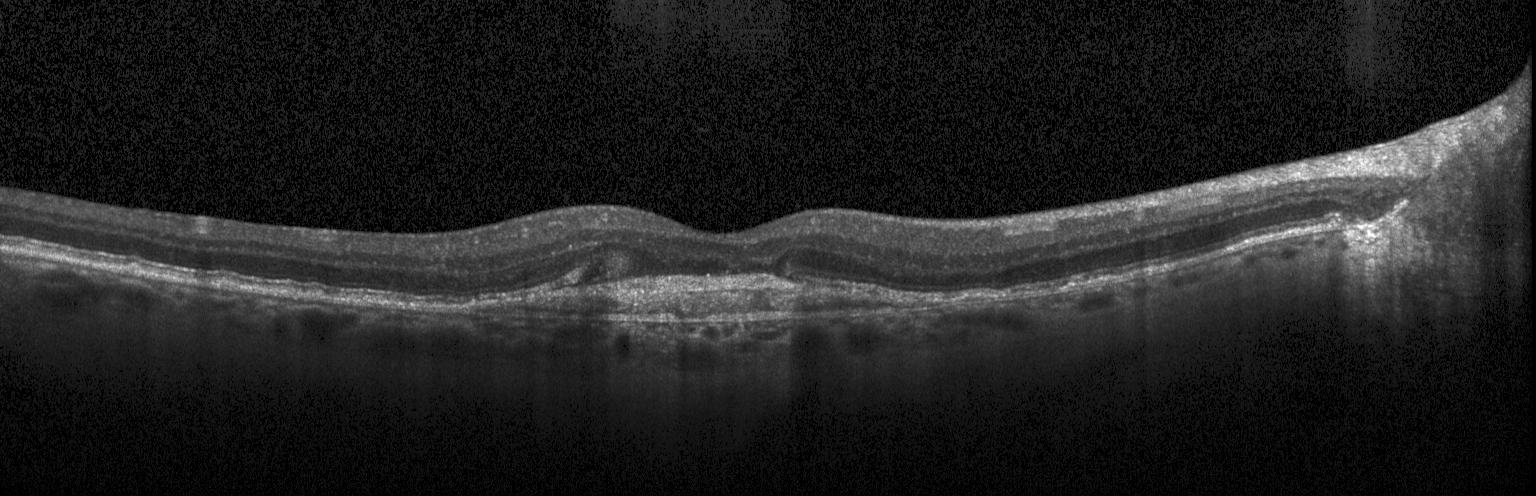 Optical coherence tomography B-scan; SD-OCT; fovea-centered; Heidelberg Spectralis OCT system. The scan shows choroidal neovascularization.